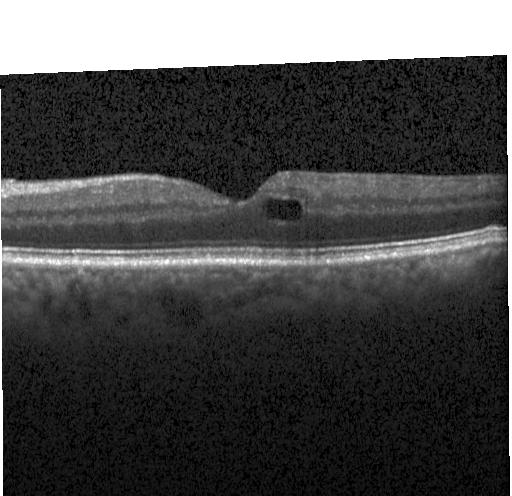

Optical coherence tomography B-scan, centered on the fovea. This B-scan demonstrates diabetic macular edema.